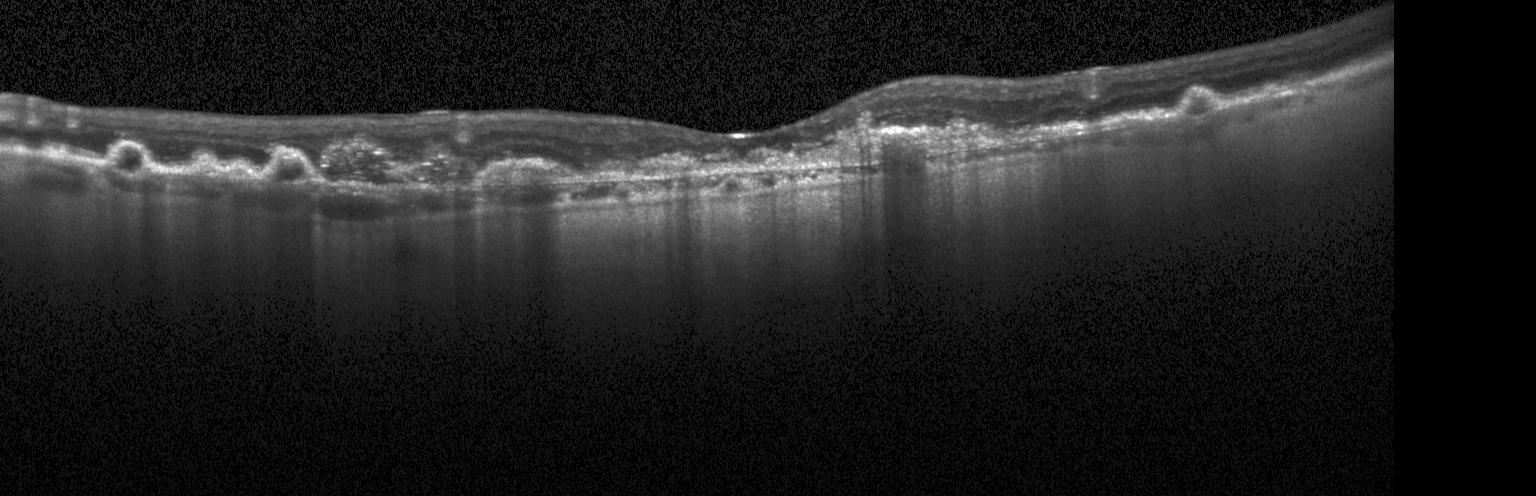
OCT finding: a choroidal neovascular membrane.